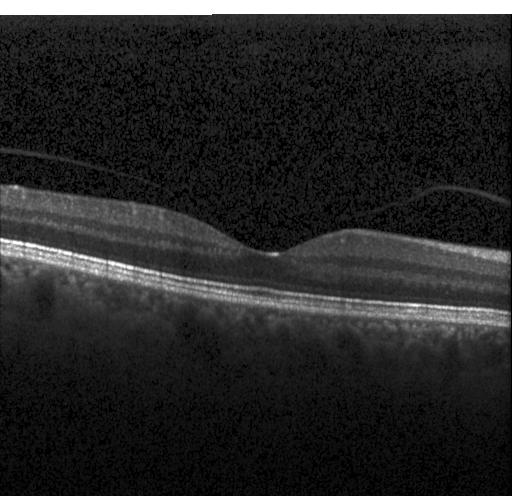

Macular scan; acquired on a Heidelberg Spectralis; OCT line scan.
This B-scan demonstrates no CNV, DME, or drusen.